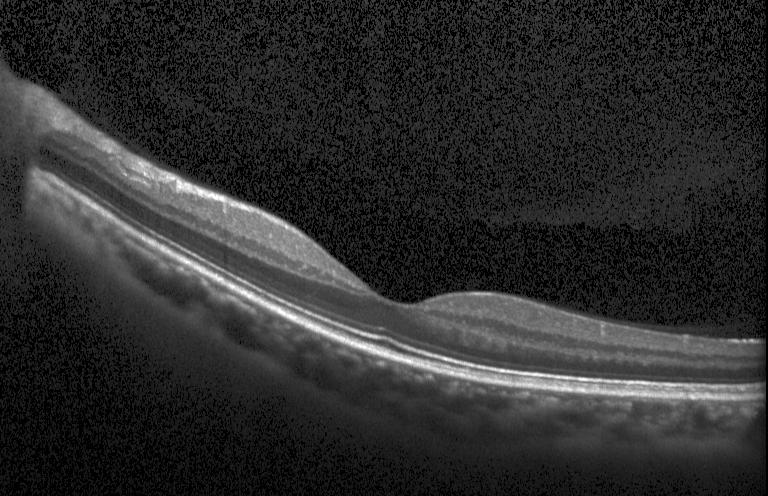
Horizontal scan through the fovea. Heidelberg Spectralis OCT system. Retinal OCT B-scan. Spectral-domain optical coherence tomography. This B-scan demonstrates neither CNV, DME, nor drusen.